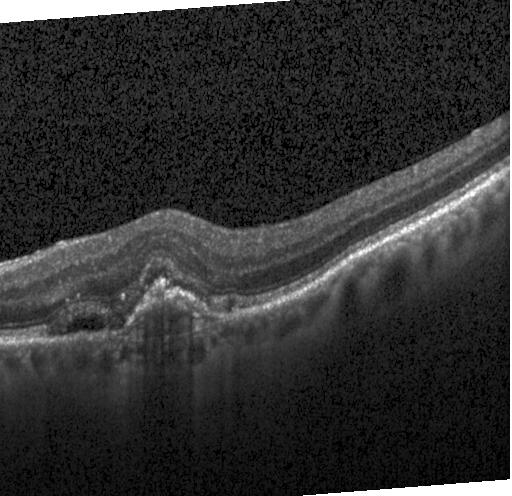

Dx: a choroidal neovascular membrane.